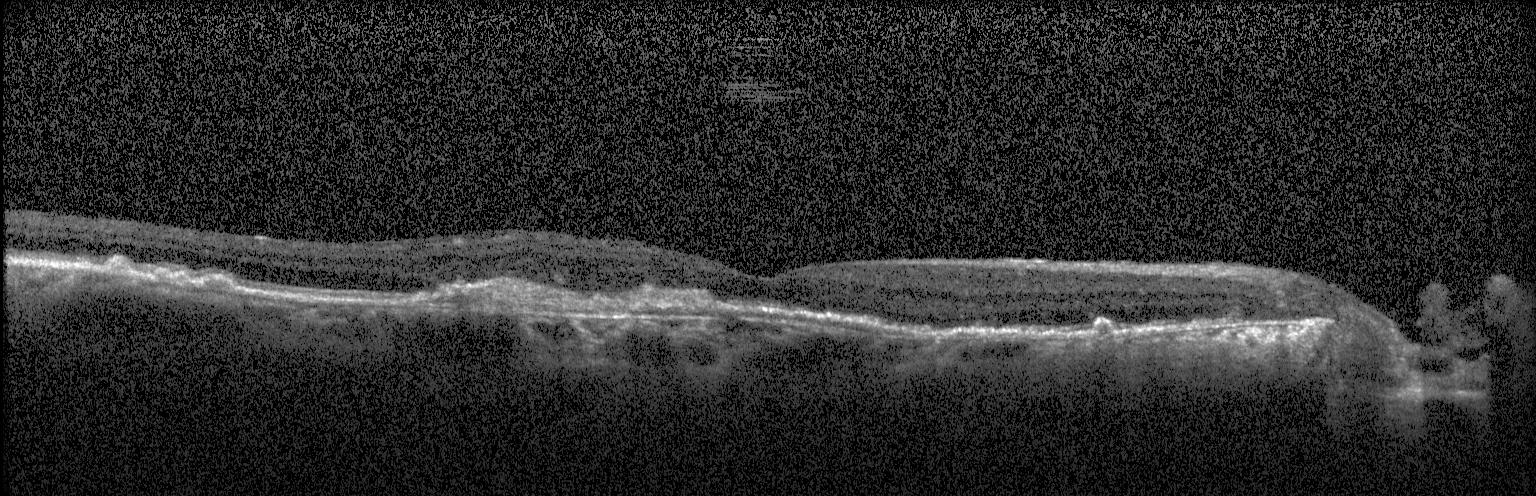 Optical coherence tomography B-scan; spectral-domain OCT.
Finding: CNV.